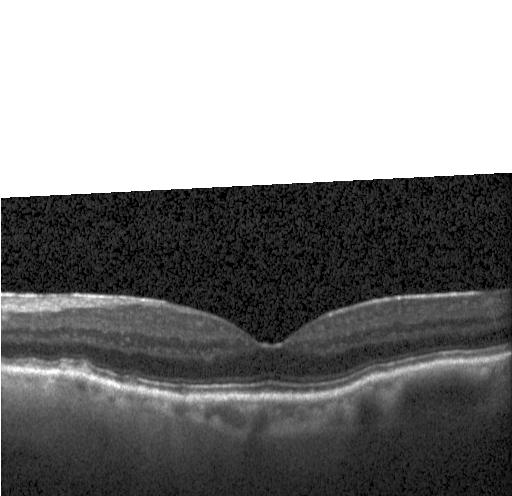 OCT line scan; centered on the fovea; instrument: Heidelberg Spectralis; SD-OCT. This B-scan demonstrates multiple drusen.